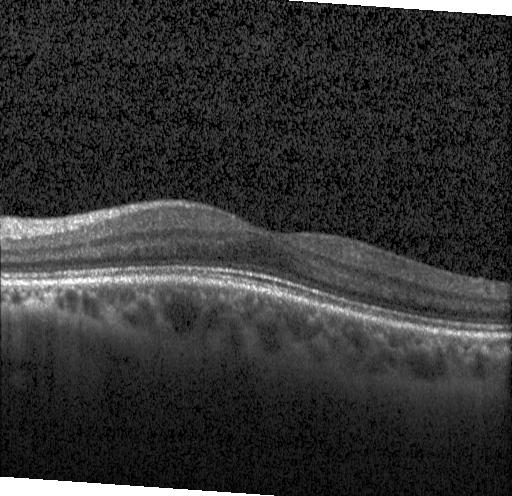

Finding: neither choroidal neovascularization, diabetic macular edema, nor drusen.